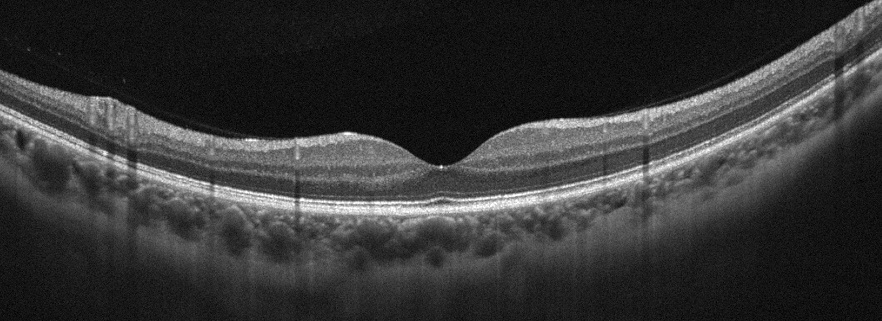 Retinal OCT cross-section showing no AMD, DME, ERM, RAO, RVO, or VID.